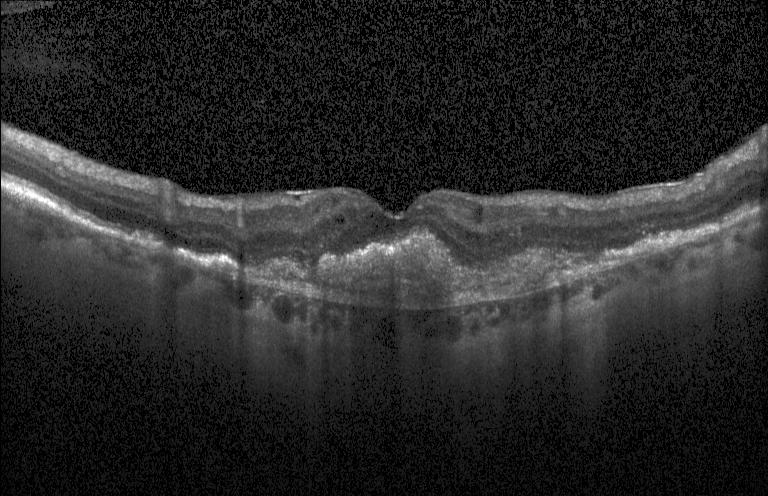
Spectral-domain OCT · instrument: Heidelberg Spectralis · retinal OCT B-scan · through the macula
Macular OCT: a choroidal neovascular membrane.